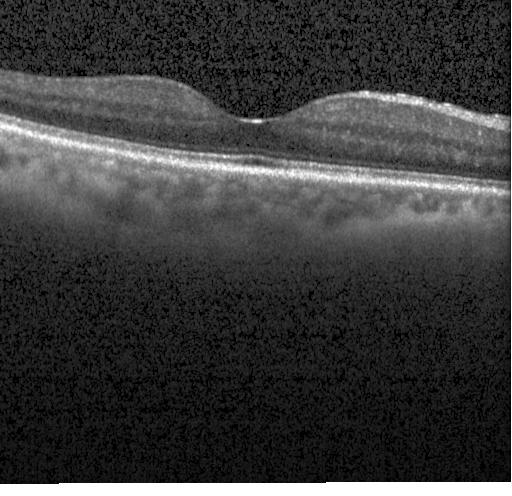
Macular scan, retinal OCT cross-section, acquired on a Heidelberg Spectralis. Finding: no CNV, DME, or drusen.